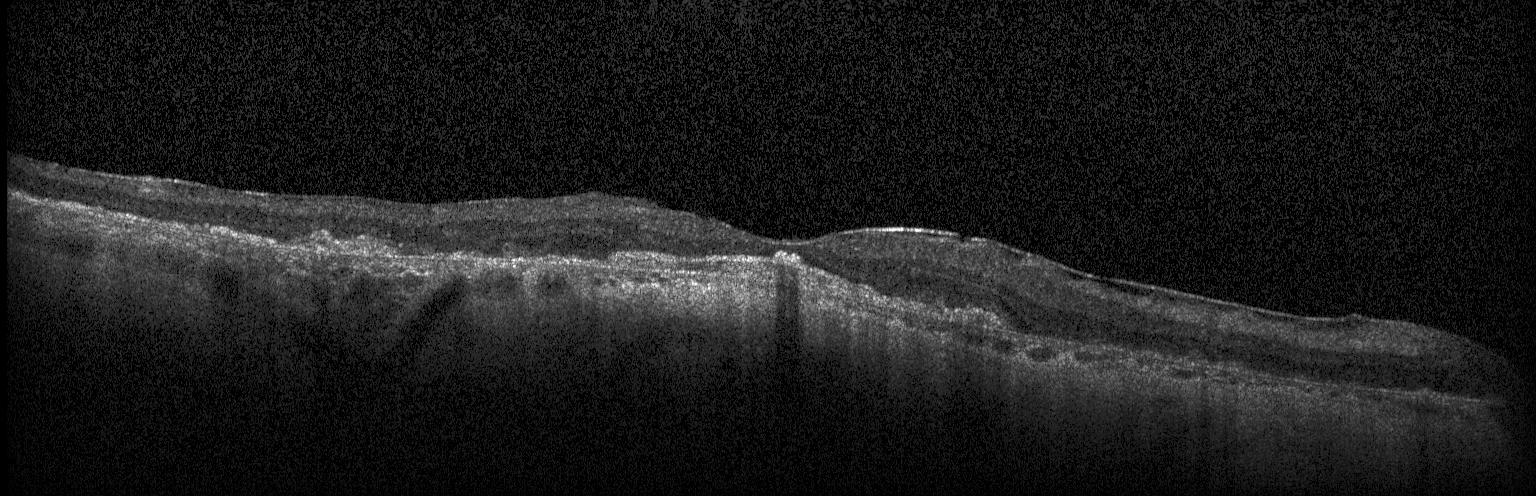
Heidelberg Spectralis OCT system · OCT line scan · macular scan — A choroidal neovascular membrane.